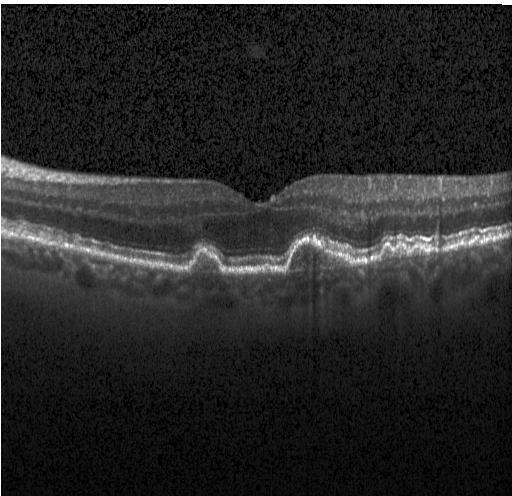
Drusen.